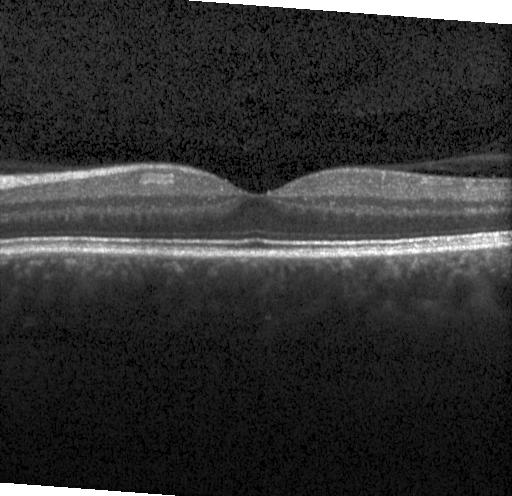
Through the macula; spectral-domain optical coherence tomography; acquired on a Heidelberg Spectralis; optical coherence tomography scan. Diagnosis: neither CNV, DME, nor drusen.